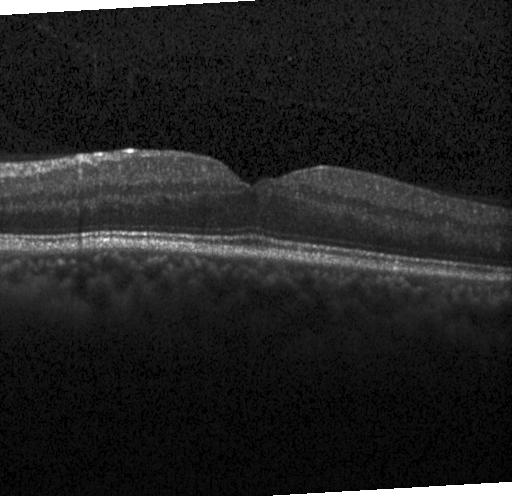

Dx: no choroidal neovascularization, diabetic macular edema, or drusen.